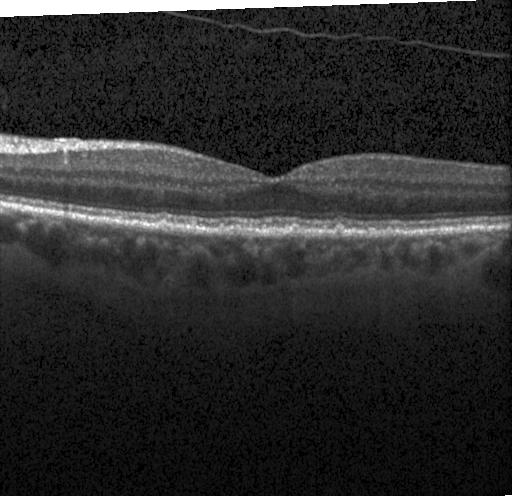
Diagnosis: drusen.